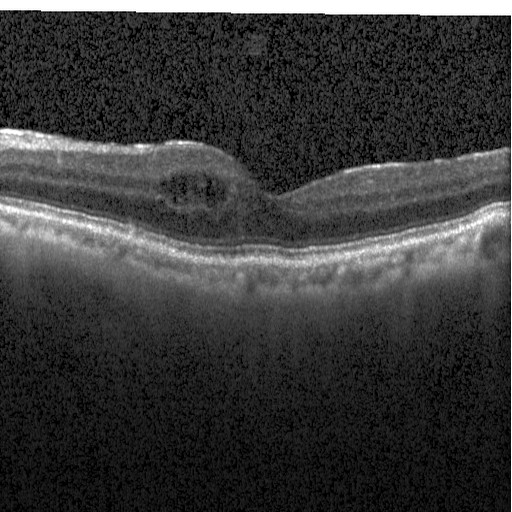

Retinal OCT B-scan.
Diagnosis: DME.